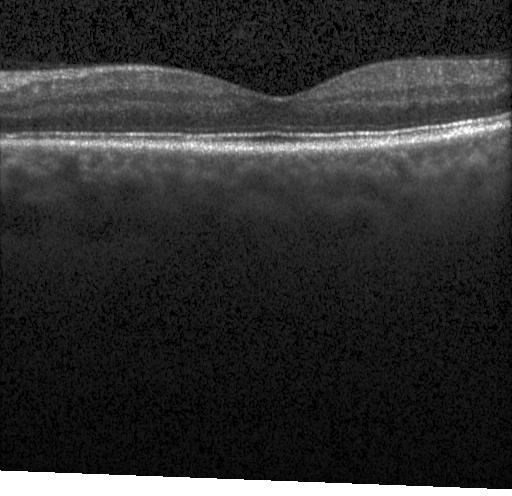

Optical coherence tomography scan — No evidence of choroidal neovascularization, diabetic macular edema, or drusen.